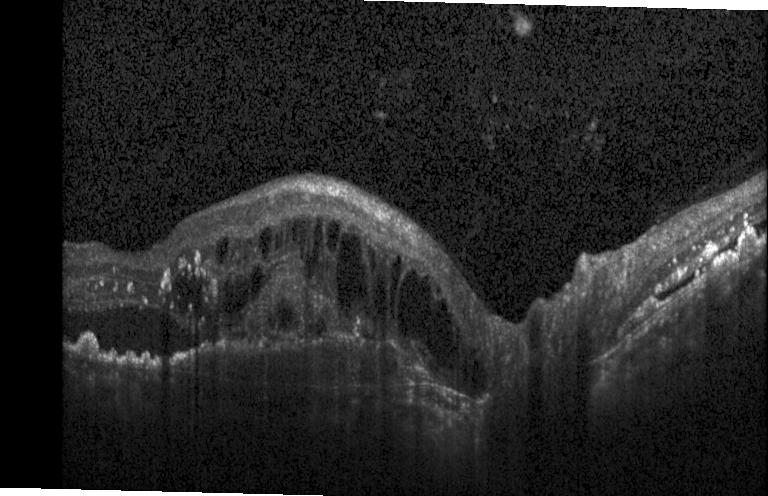

Macular OCT demonstrating CNV.